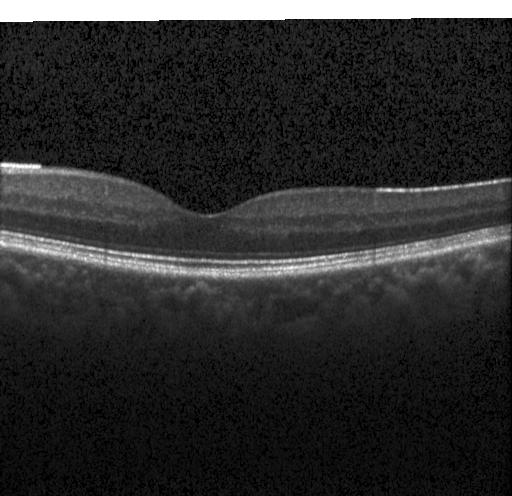

Optical coherence tomography scan · spectral-domain optical coherence tomography.
Diagnosis: no evidence of choroidal neovascularization, diabetic macular edema, or drusen.